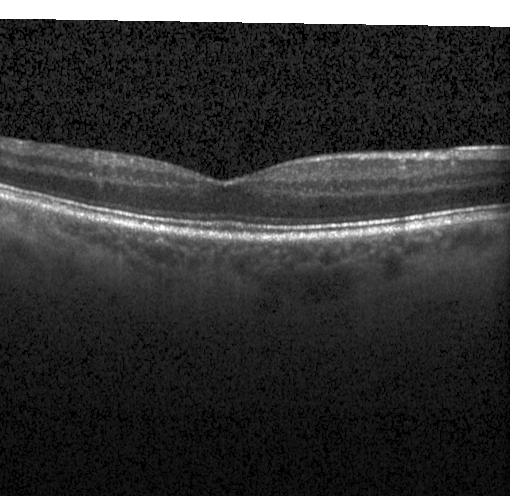
OCT B-scan; centered on the fovea. Diagnosis: no evidence of choroidal neovascularization, diabetic macular edema, or drusen.